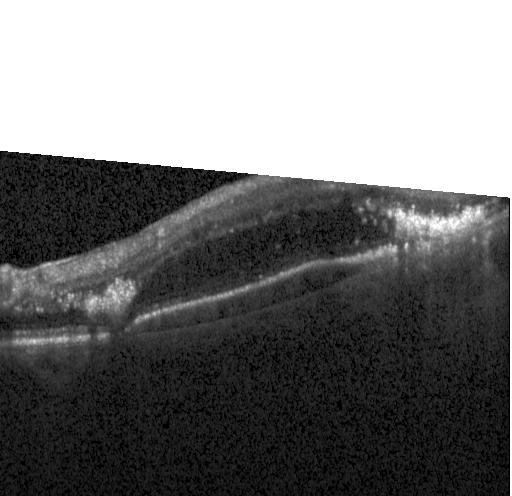
Retinal OCT B-scan.
Finding: diabetic macular edema.